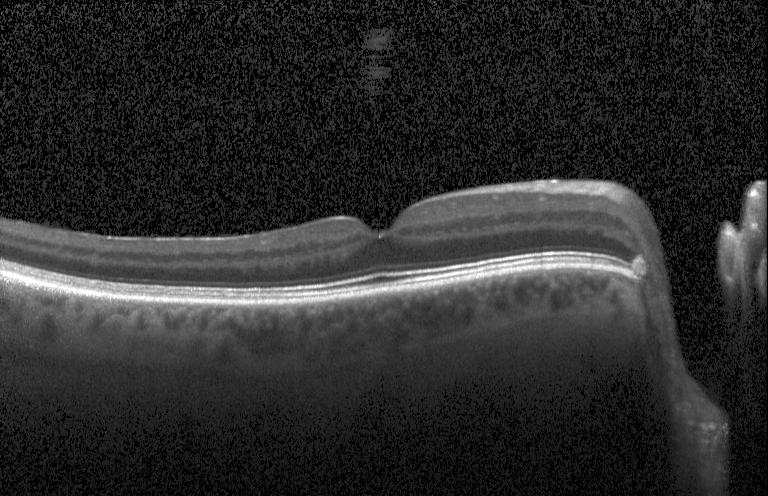 Retinal OCT cross-section showing neither choroidal neovascularization, diabetic macular edema, nor drusen.